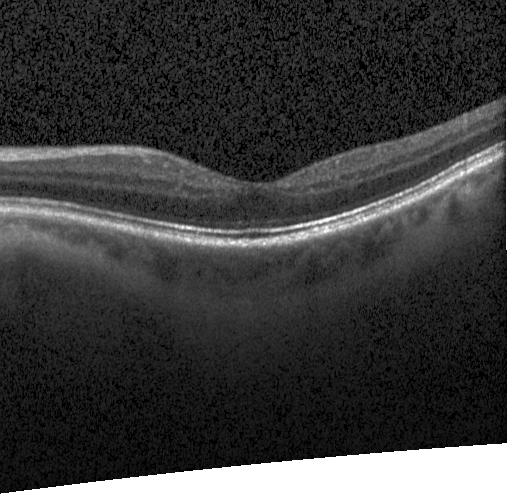
Retinal OCT cross-section showing no evidence of choroidal neovascularization, diabetic macular edema, or drusen.